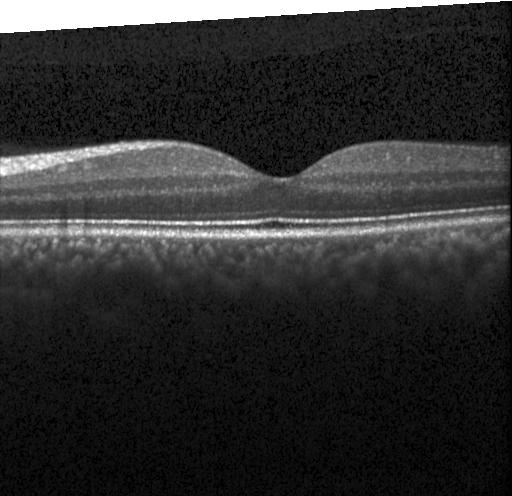

Optical coherence tomography B-scan
Macular OCT: no choroidal neovascularization, diabetic macular edema, or drusen.